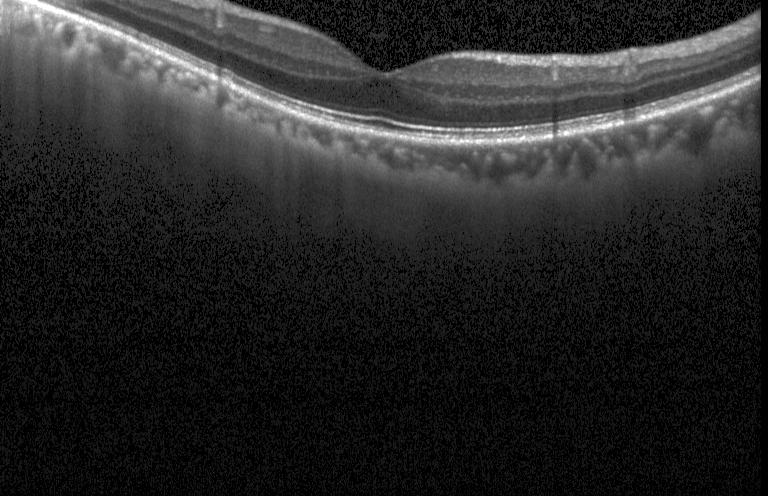 Impression: no evidence of choroidal neovascularization, diabetic macular edema, or drusen.